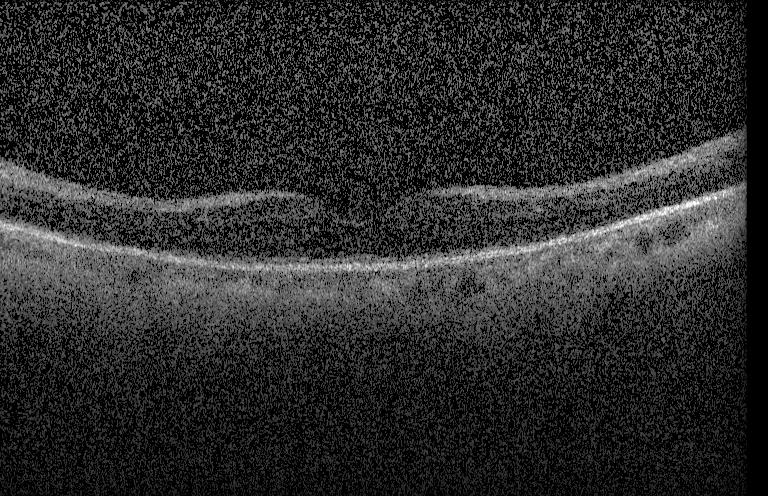

Retinal OCT B-scan. Impression: no evidence of choroidal neovascularization, diabetic macular edema, or drusen.